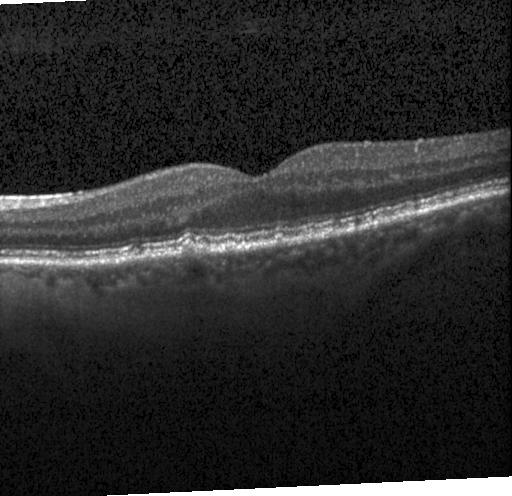
Optical coherence tomography B-scan. Through the macula. Acquired on a Heidelberg Spectralis. SD-OCT.
Dx: multiple drusen.